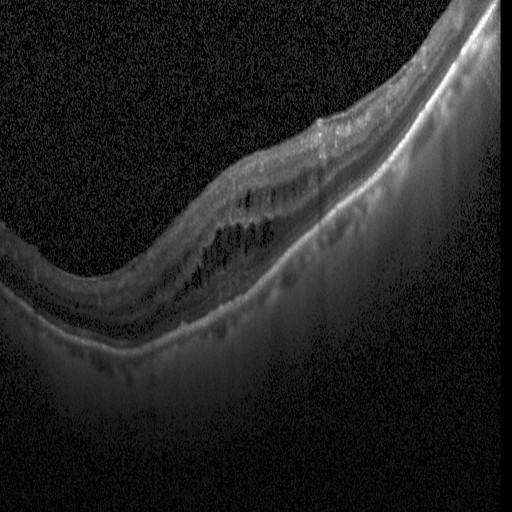 Instrument: Heidelberg Spectralis · optical coherence tomography scan · through the macula — Finding: diabetic macular edema (DME).